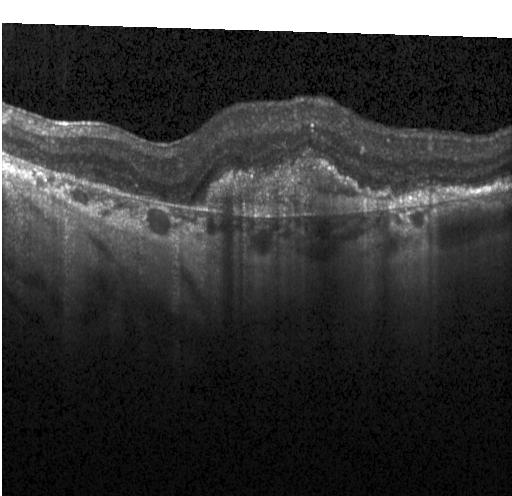

Optical coherence tomography B-scan
A choroidal neovascular membrane.